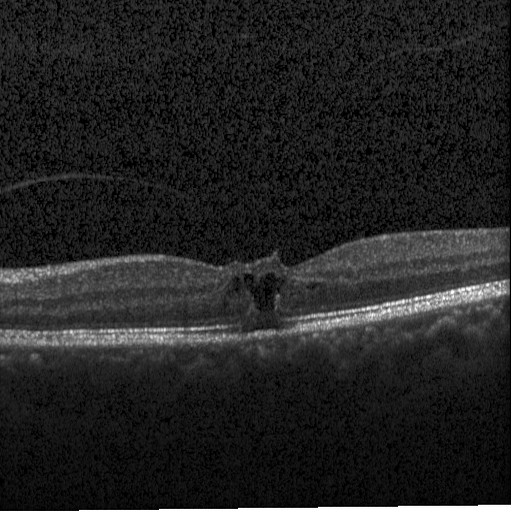 Optical coherence tomography B-scan, SD-OCT, acquired on a Heidelberg Spectralis, macular scan — This B-scan demonstrates DME.